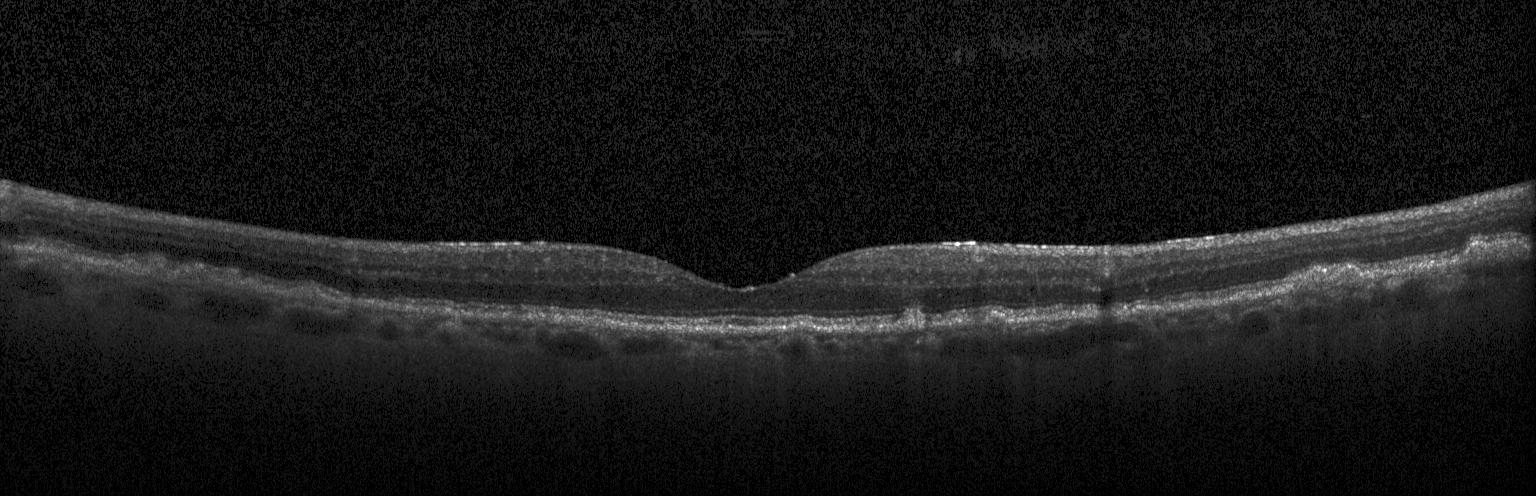

OCT B-scan
Diagnosis: drusen.